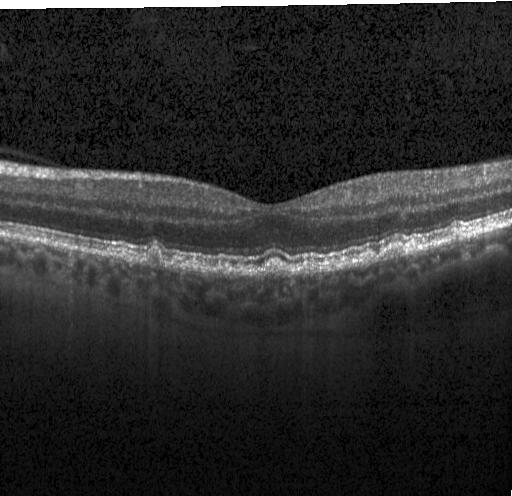

Through the macula. Spectral-domain optical coherence tomography. Optical coherence tomography B-scan. Acquired on a Heidelberg Spectralis. Impression: multiple drusen.